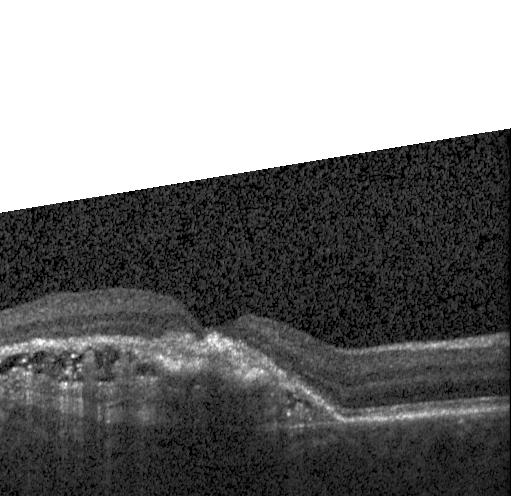
OCT line scan, Heidelberg Spectralis, SD-OCT
Finding: CNV.